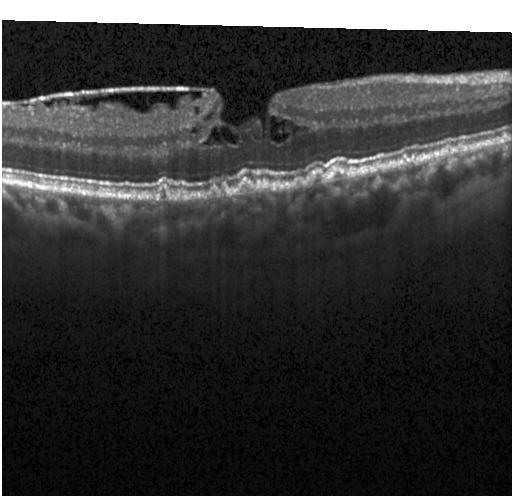 Acquired on a Heidelberg Spectralis; OCT B-scan. Drusen.